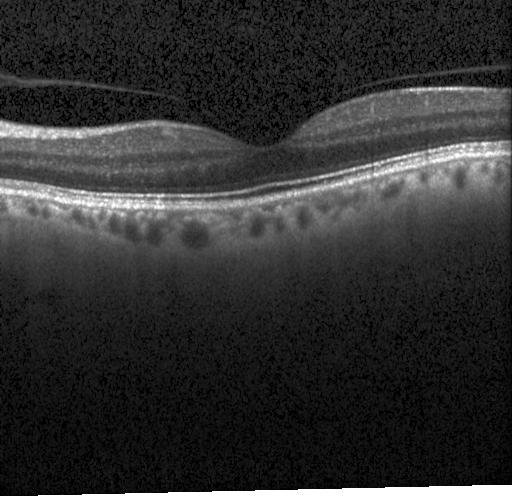

Diagnosis: neither choroidal neovascularization, diabetic macular edema, nor drusen.